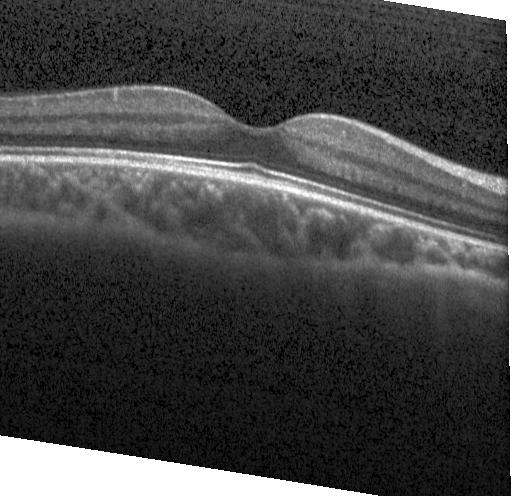

Retinal OCT B-scan — Finding: no CNV, no DME, and no drusen.